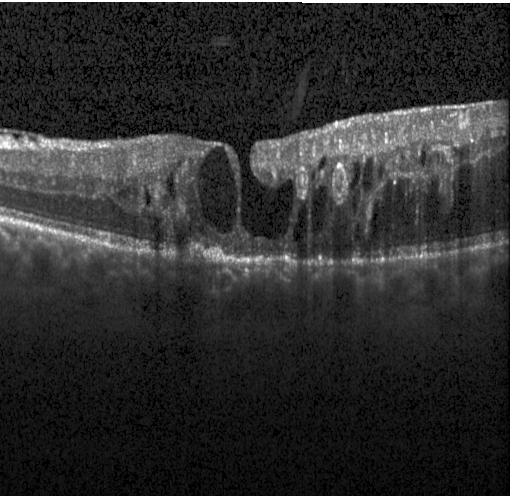

OCT scan showing diabetic macular edema (DME).